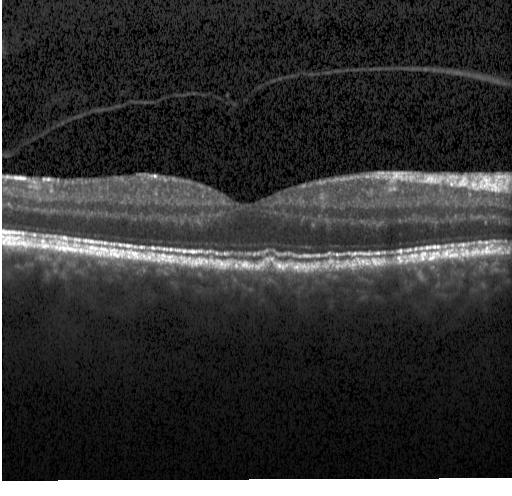 OCT B-scan. Centered on the fovea. Acquired on a Heidelberg Spectralis
Drusen.